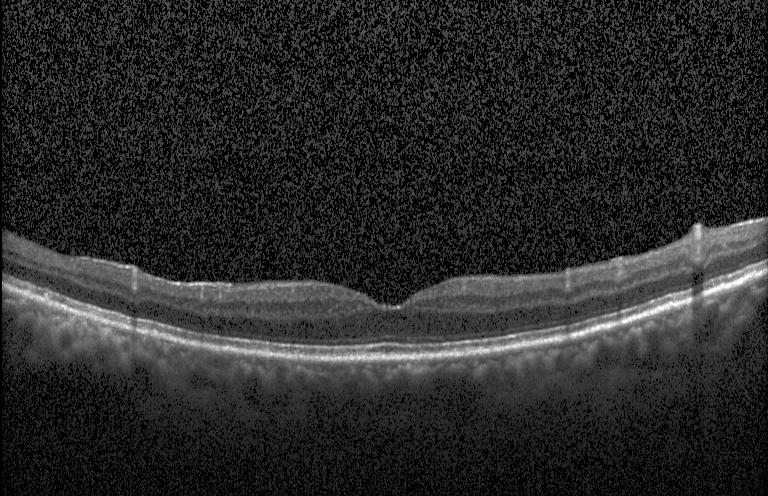

Acquired on a Heidelberg Spectralis; OCT line scan; through the macula. Finding: no choroidal neovascularization, no diabetic macular edema, and no drusen.